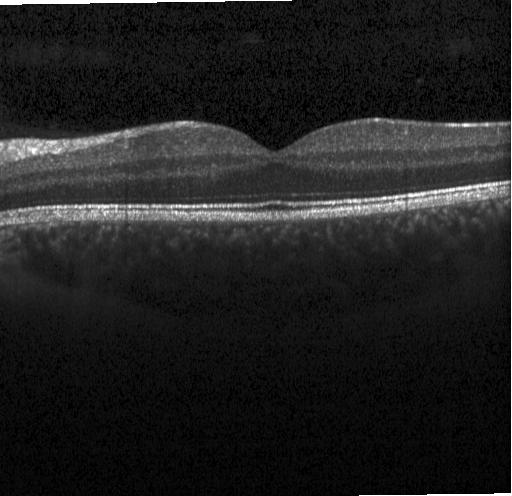 Retinal OCT cross-section. Through the macula. Instrument: Heidelberg Spectralis — Impression: neither choroidal neovascularization, diabetic macular edema, nor drusen.